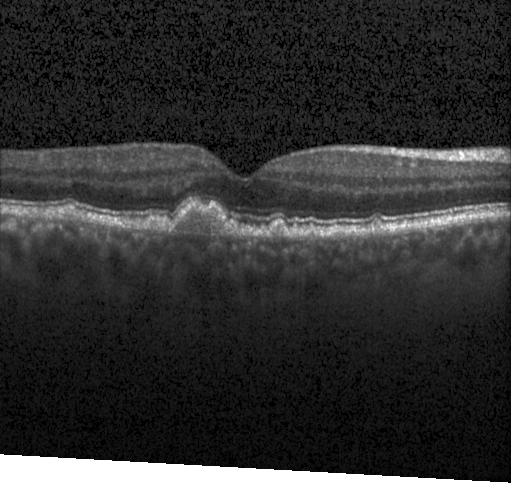
Retinal OCT cross-section showing a choroidal neovascular membrane.